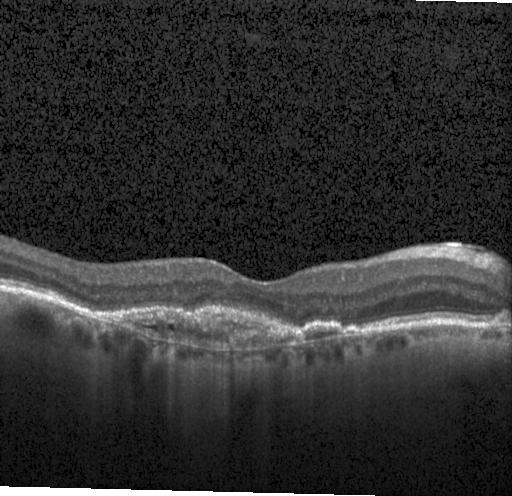

OCT line scan. Impression: CNV.